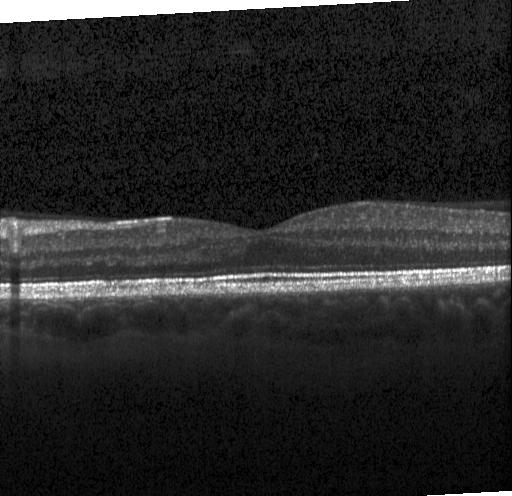

Acquired on a Heidelberg Spectralis, spectral-domain optical coherence tomography, macular scan, optical coherence tomography scan.
Diagnosis: neither CNV, DME, nor drusen.